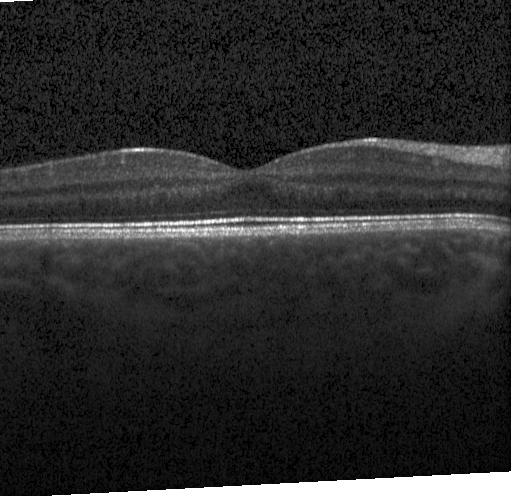
Diagnosis: no choroidal neovascularization, diabetic macular edema, or drusen.